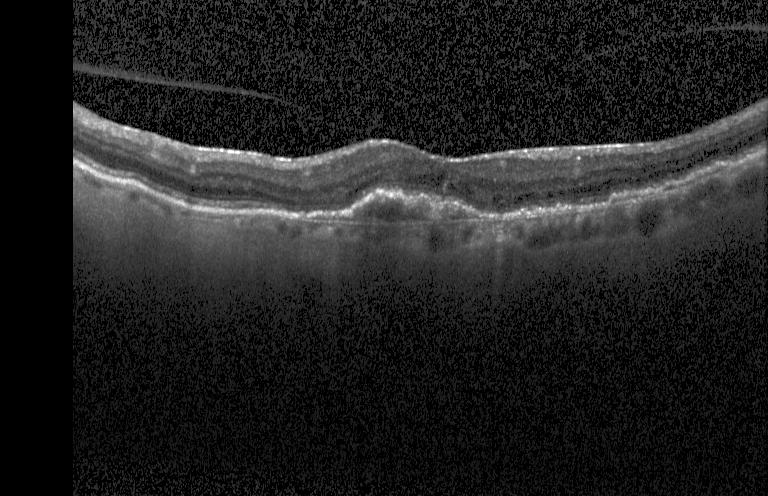 Acquired on a Heidelberg Spectralis; retinal OCT cross-section; through the macula; spectral-domain optical coherence tomography
Dx: choroidal neovascularization (CNV).